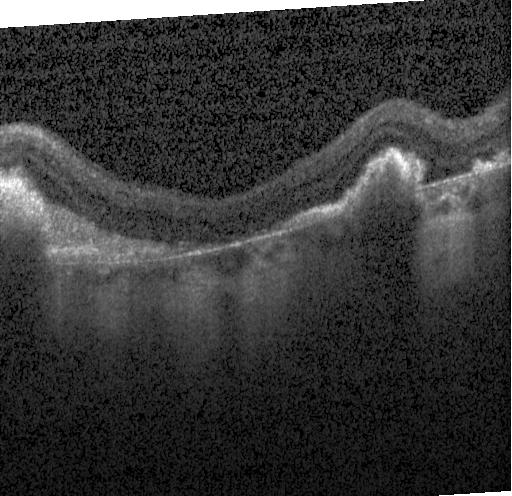
Retinal OCT B-scan
The scan shows a choroidal neovascular membrane.